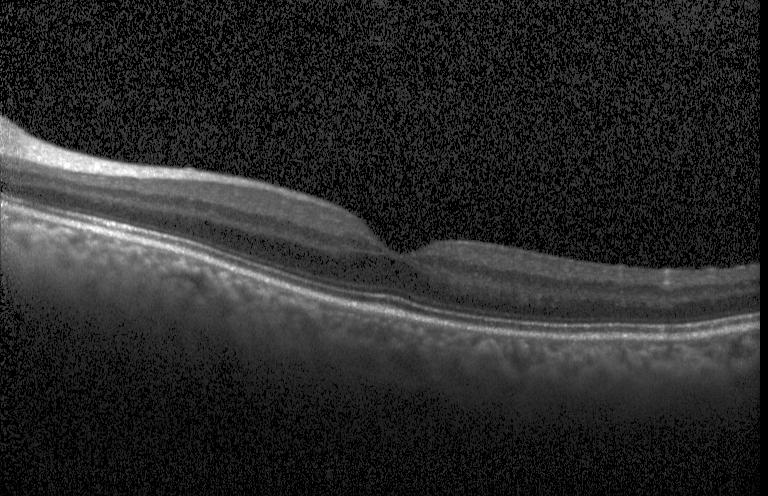

Acquired on a Heidelberg Spectralis · optical coherence tomography B-scan · through the macula · spectral-domain OCT.
No evidence of choroidal neovascularization, diabetic macular edema, or drusen.